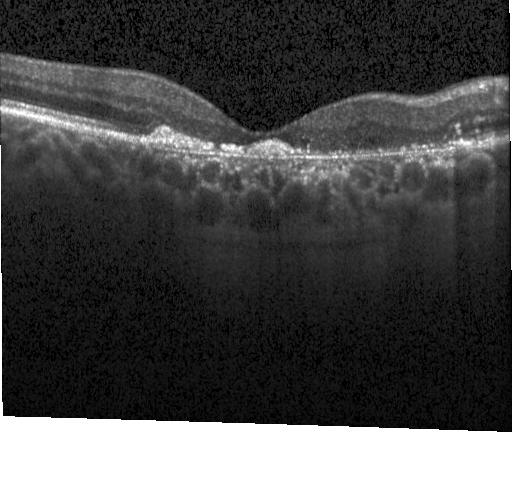
Centered on the fovea · SD-OCT · Heidelberg Spectralis · OCT line scan — Finding: CNV.